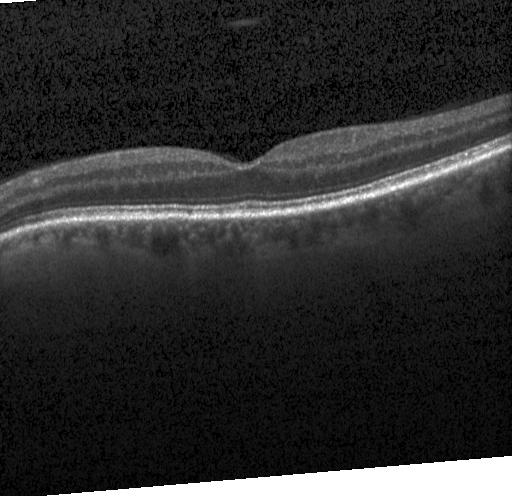

Impression: neither CNV, DME, nor drusen.